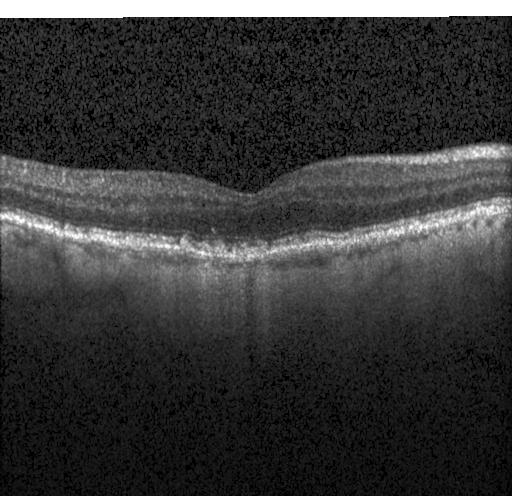
Finding: sub-RPE drusenoid deposits.